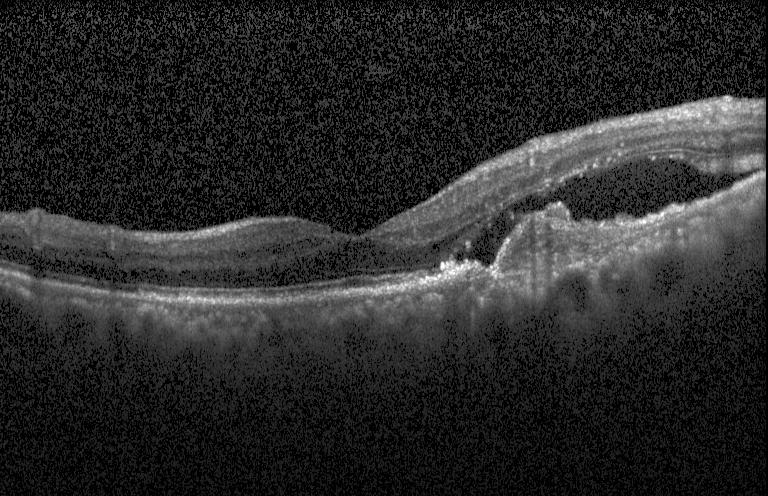 Optical coherence tomography B-scan — Impression: a choroidal neovascular membrane.